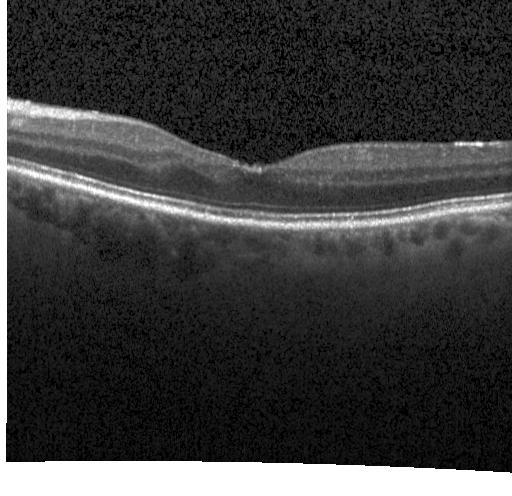

Spectral-domain OCT. OCT B-scan. Heidelberg Spectralis. Horizontal scan through the fovea. Diagnosis: neither choroidal neovascularization, diabetic macular edema, nor drusen.